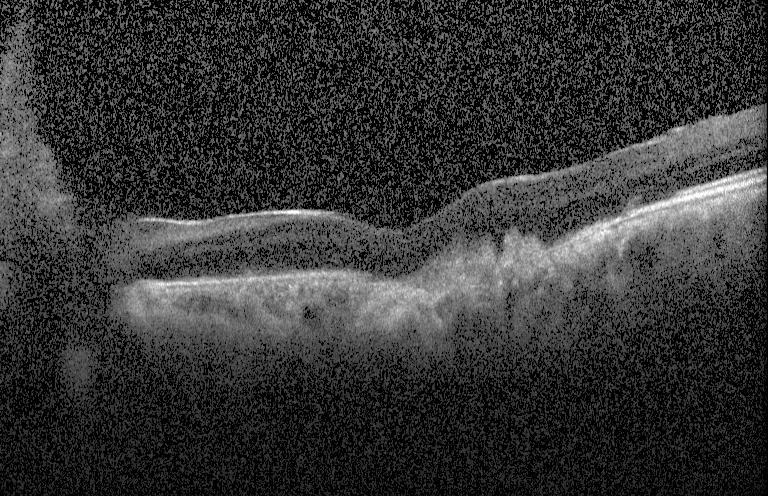

Diagnosis: CNV.